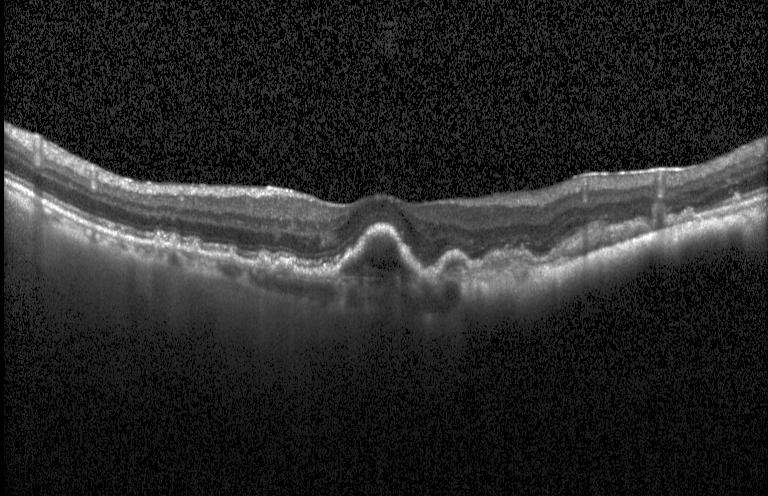
Retinal OCT cross-section. This B-scan demonstrates CNV.